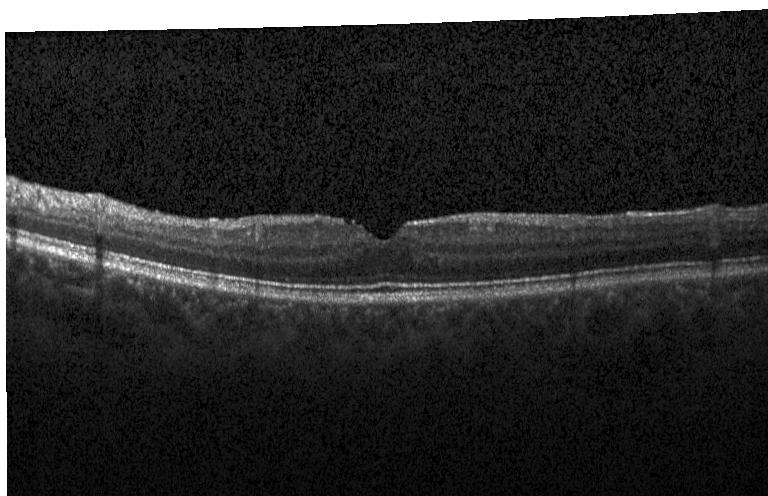
Macular OCT demonstrating no CNV, no DME, and no drusen.